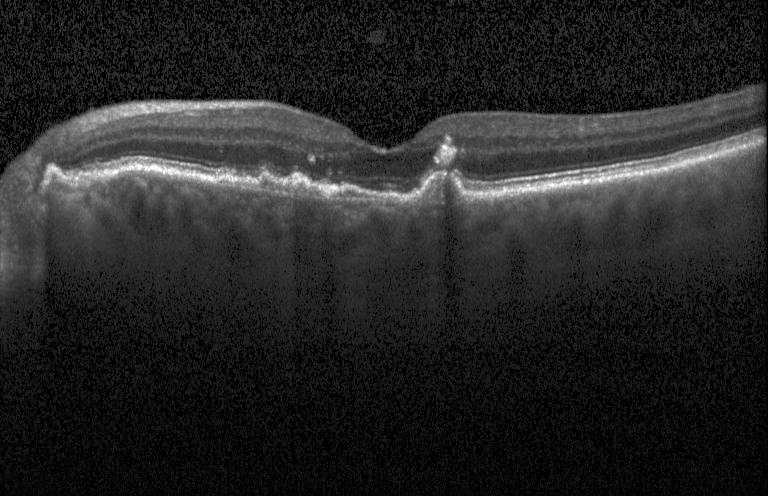

Acquired on a Heidelberg Spectralis; centered on the fovea; OCT B-scan; SD-OCT — The scan shows a choroidal neovascular membrane.